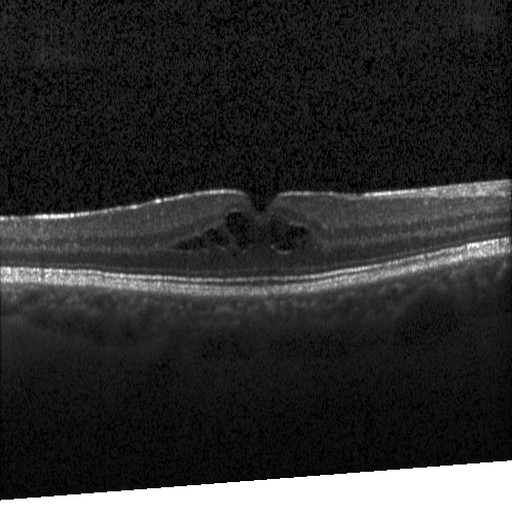 Impression: DME.